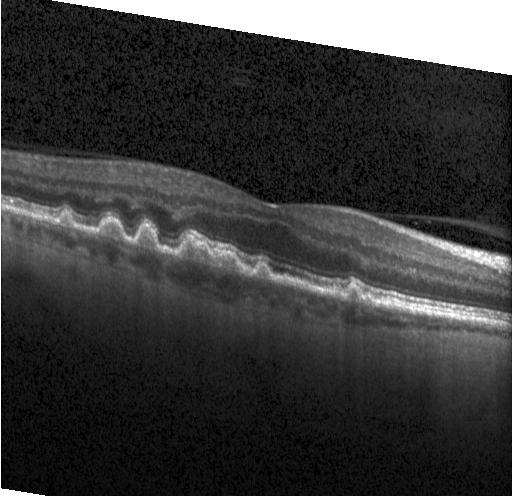
This B-scan demonstrates sub-RPE drusenoid deposits.